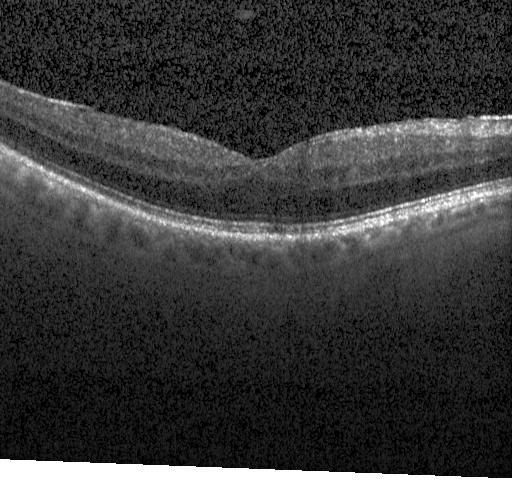

SD-OCT. Centered on the fovea. OCT B-scan. Heidelberg Spectralis OCT system.
Dx: no choroidal neovascularization, diabetic macular edema, or drusen.